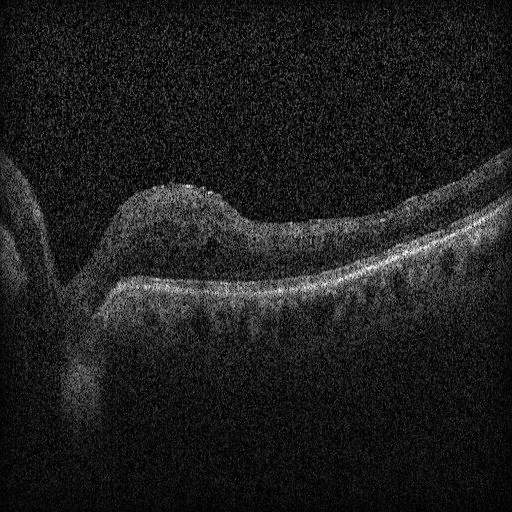

Retinal OCT cross-section.
Diagnosis: diabetic macular edema.